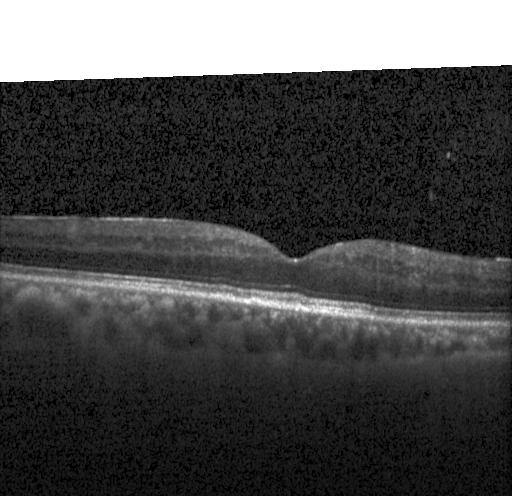

Finding: neither CNV, DME, nor drusen.